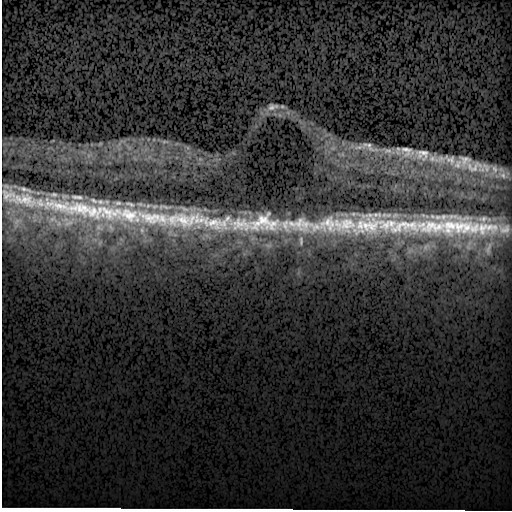

OCT line scan. This B-scan demonstrates diabetic macular edema.